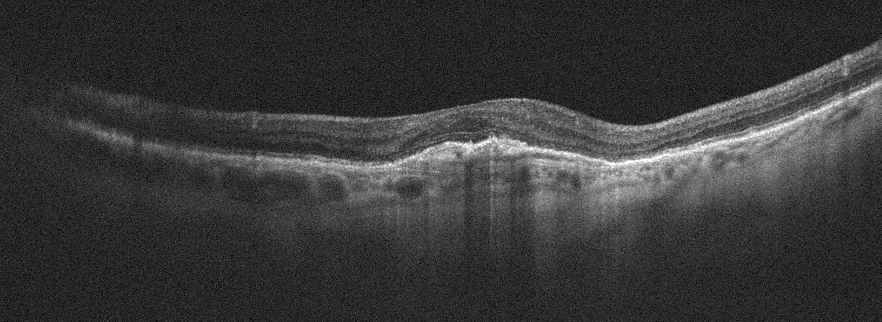
OCT line scan.
Assessment: age-related macular degeneration (AMD).